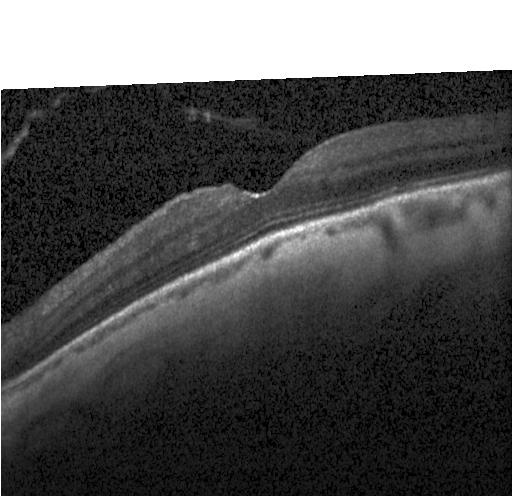

Impression: no choroidal neovascularization, no diabetic macular edema, and no drusen.